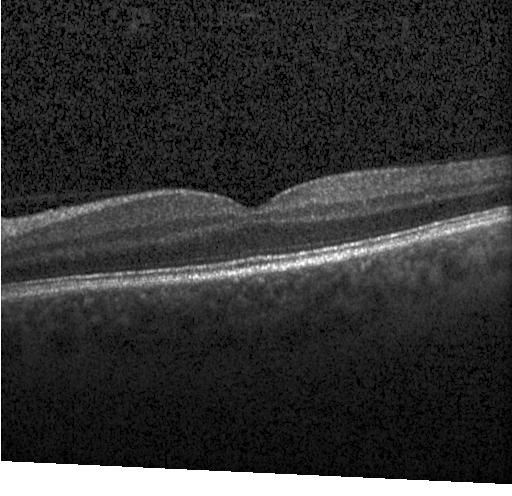 OCT B-scan; horizontal scan through the fovea; acquired on a Heidelberg Spectralis. Finding: no choroidal neovascularization, no diabetic macular edema, and no drusen.